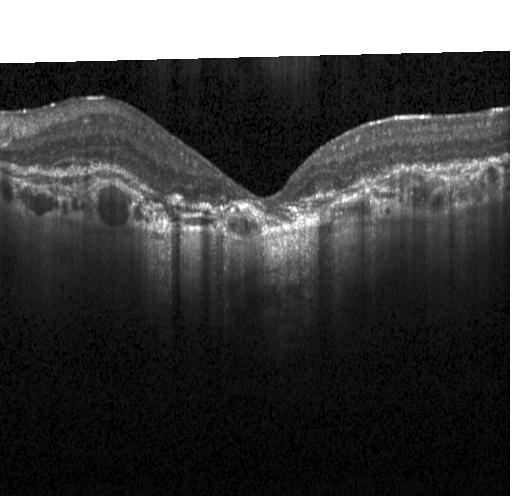

Heidelberg Spectralis OCT system · optical coherence tomography B-scan — OCT finding: choroidal neovascularization.